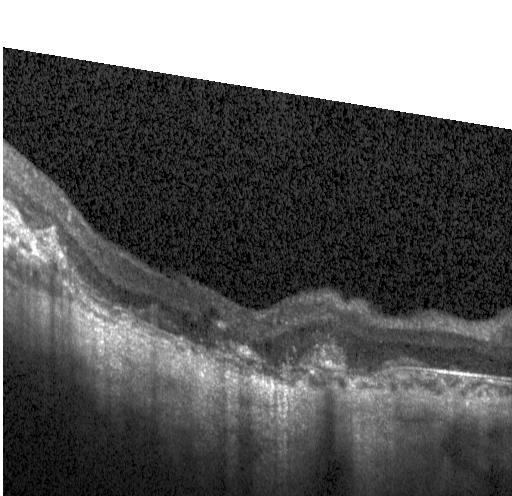
Dx: a choroidal neovascular membrane.